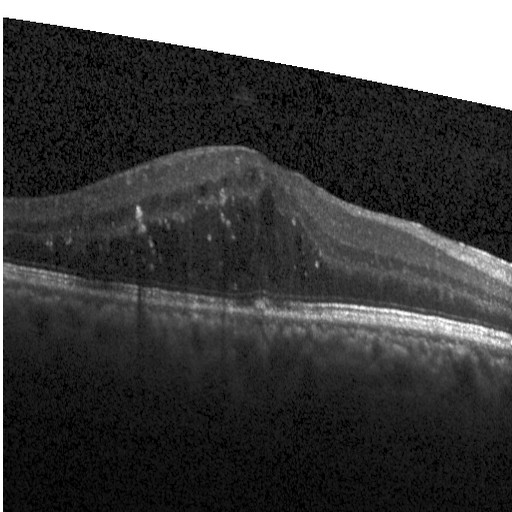 Acquired on a Heidelberg Spectralis. Horizontal scan through the fovea. Retinal OCT cross-section — Macular OCT: diabetic macular edema.